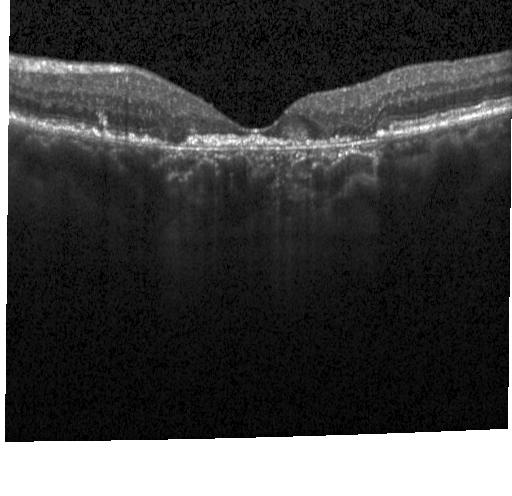
Impression: a choroidal neovascular membrane.